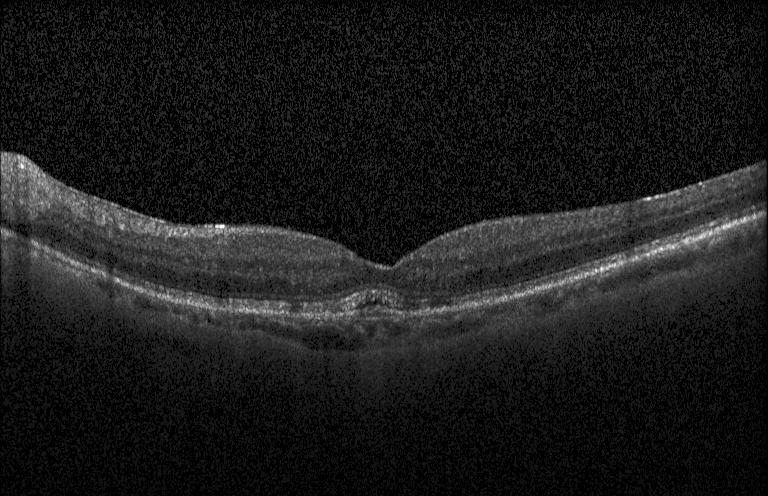
Optical coherence tomography scan
Finding: a choroidal neovascular membrane.